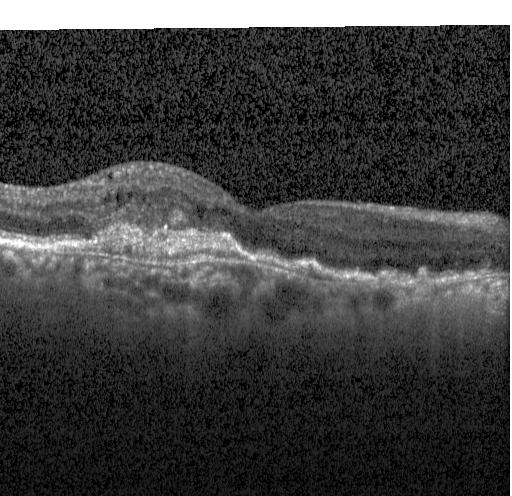 Horizontal scan through the fovea; optical coherence tomography B-scan
Finding: choroidal neovascularization (CNV).